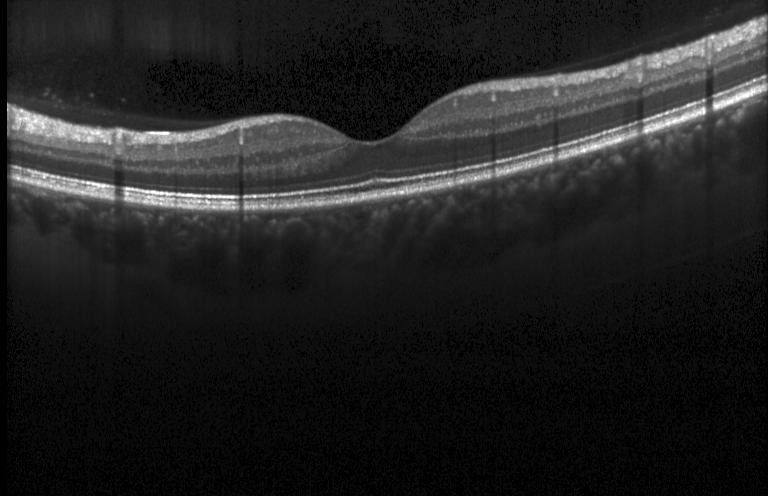
Macular OCT: neither choroidal neovascularization, diabetic macular edema, nor drusen.